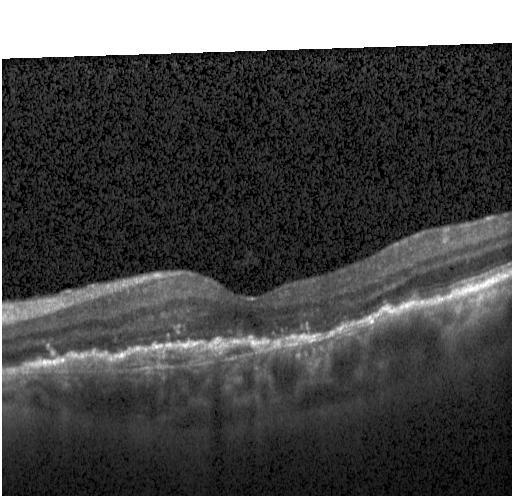 Optical coherence tomography scan. Through the macula
Dx: choroidal neovascularization.